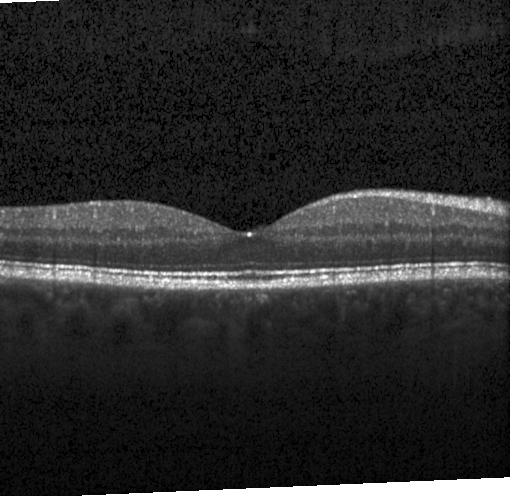

Assessment: no evidence of choroidal neovascularization, diabetic macular edema, or drusen.